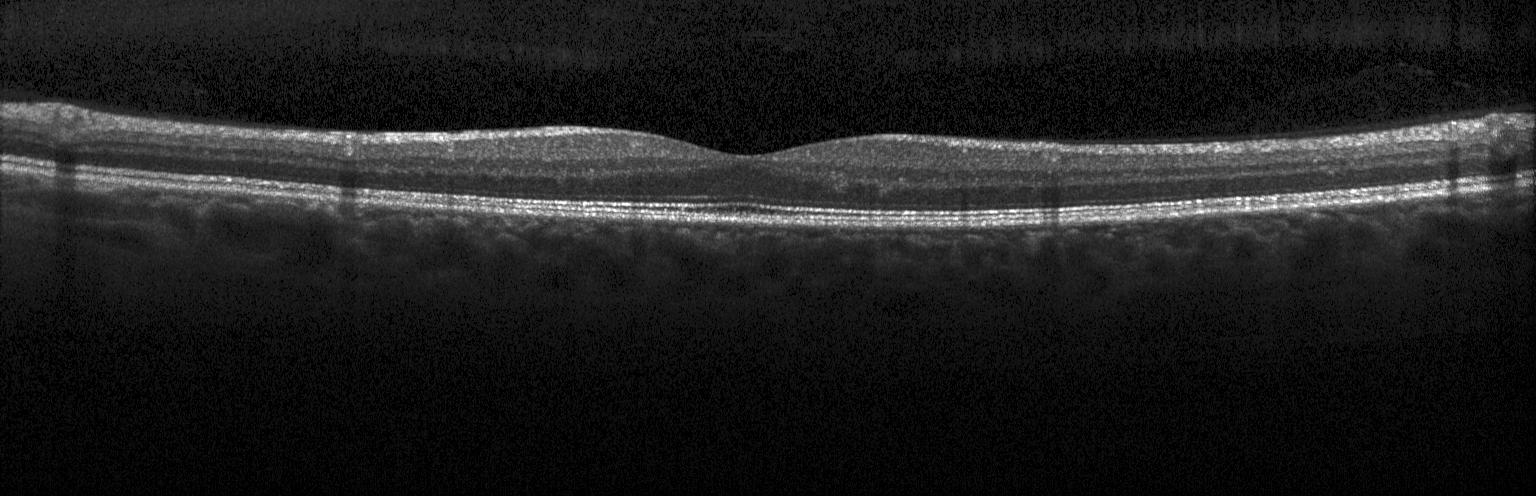 This B-scan demonstrates no evidence of choroidal neovascularization, diabetic macular edema, or drusen.